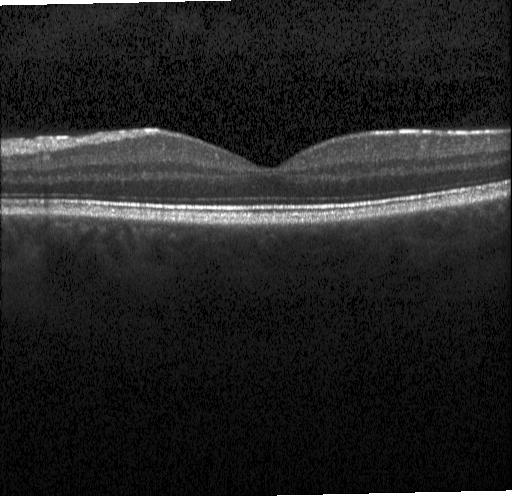 Optical coherence tomography B-scan. Dx: neither choroidal neovascularization, diabetic macular edema, nor drusen.